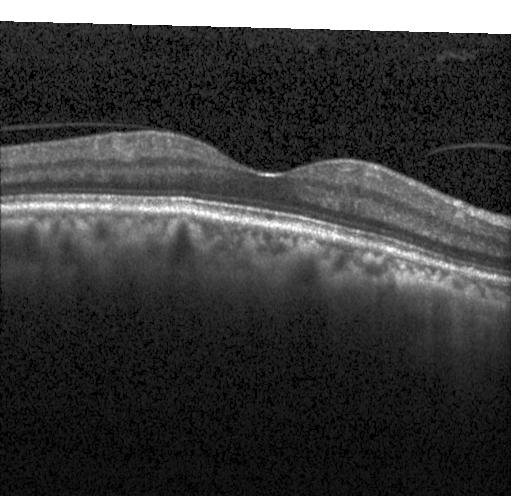

Optical coherence tomography B-scan — Impression: neither choroidal neovascularization, diabetic macular edema, nor drusen.